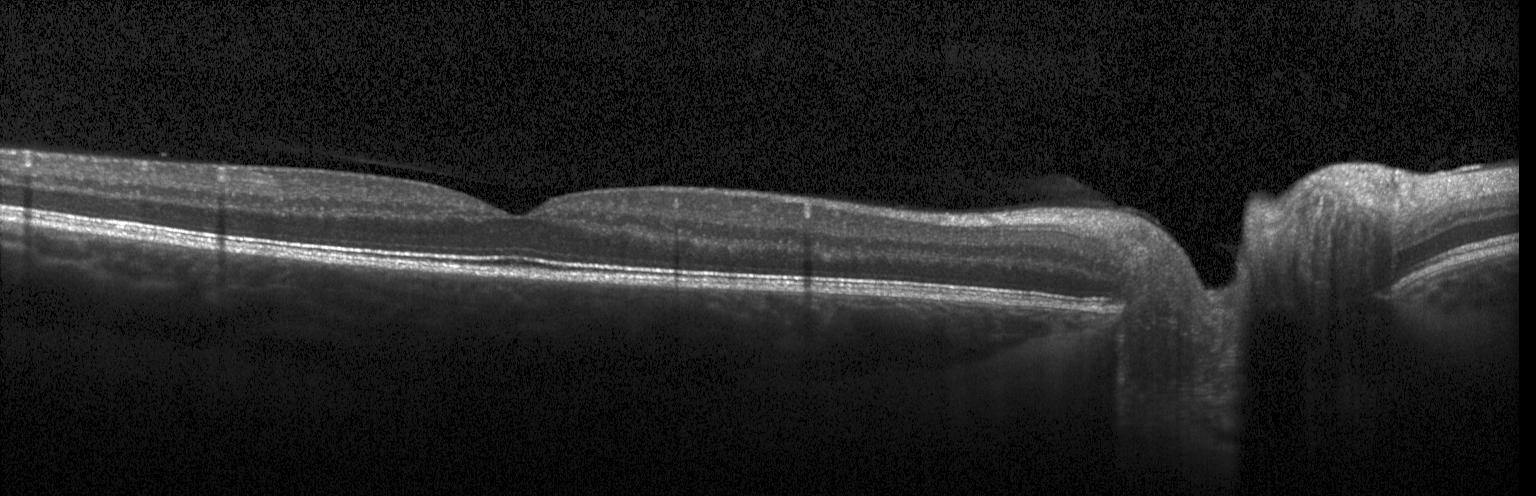
Diagnosis: neither choroidal neovascularization, diabetic macular edema, nor drusen.